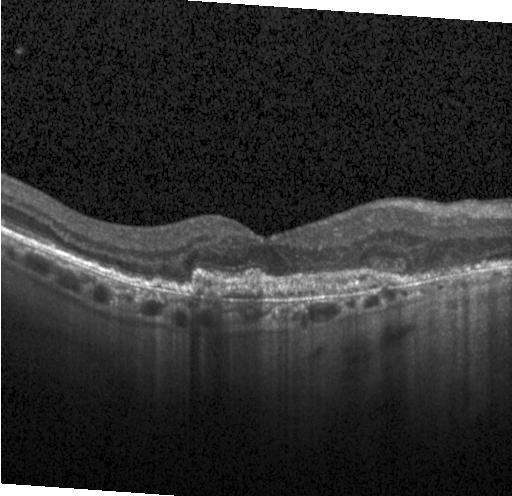 Optical coherence tomography scan — Finding: a choroidal neovascular membrane.